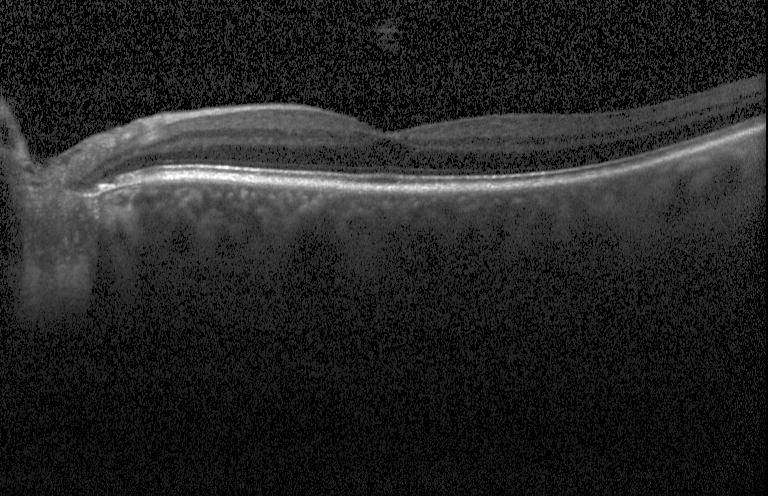 Macular OCT demonstrating neither CNV, DME, nor drusen.